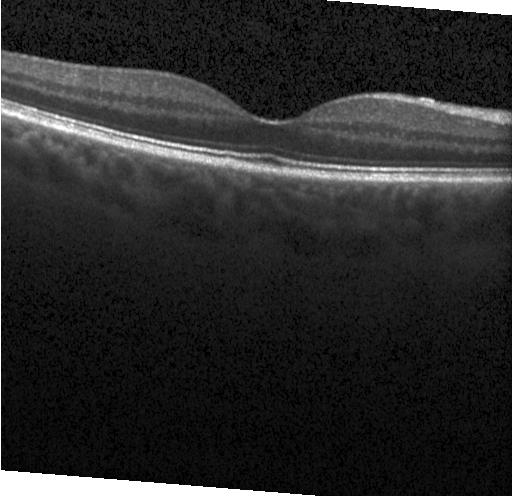

Optical coherence tomography B-scan; centered on the fovea. Macular OCT: no choroidal neovascularization, no diabetic macular edema, and no drusen.